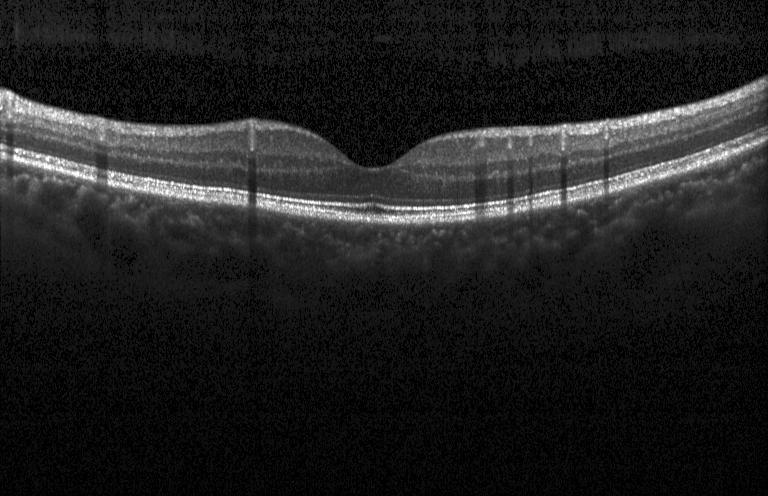 Dx: no CNV, DME, or drusen.